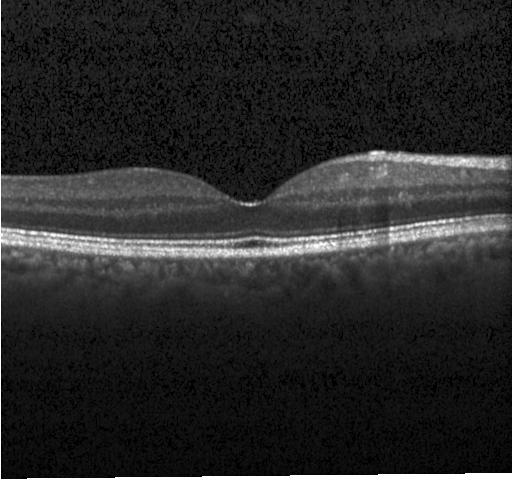
Heidelberg Spectralis, optical coherence tomography scan, fovea-centered. No choroidal neovascularization, diabetic macular edema, or drusen.